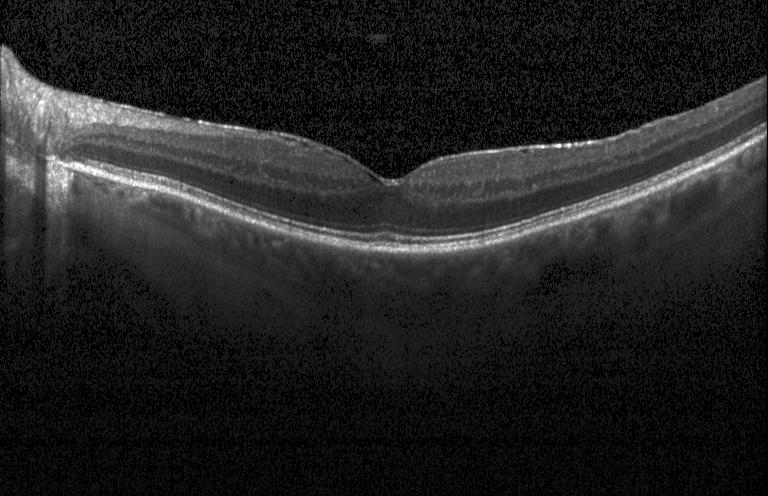 Fovea-centered. Spectral-domain optical coherence tomography. Optical coherence tomography scan
Diagnosis: neither choroidal neovascularization, diabetic macular edema, nor drusen.